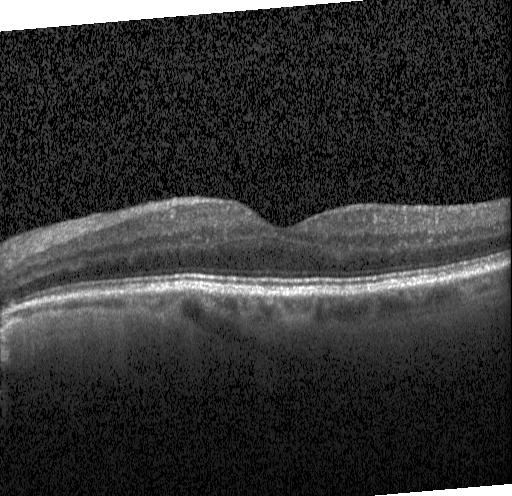
Optical coherence tomography B-scan
Finding: no CNV, no DME, and no drusen.